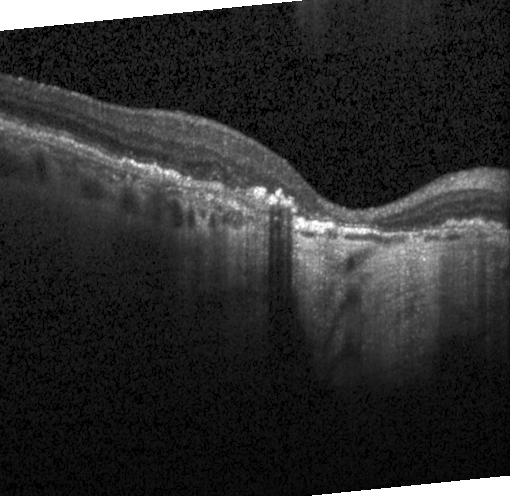

Diagnosis: CNV.